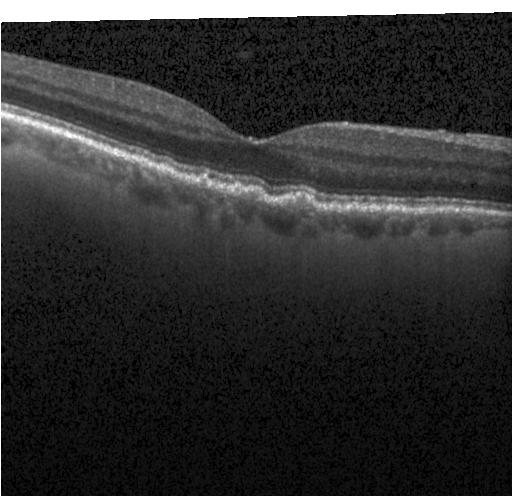 Diagnosis: sub-RPE drusenoid deposits.